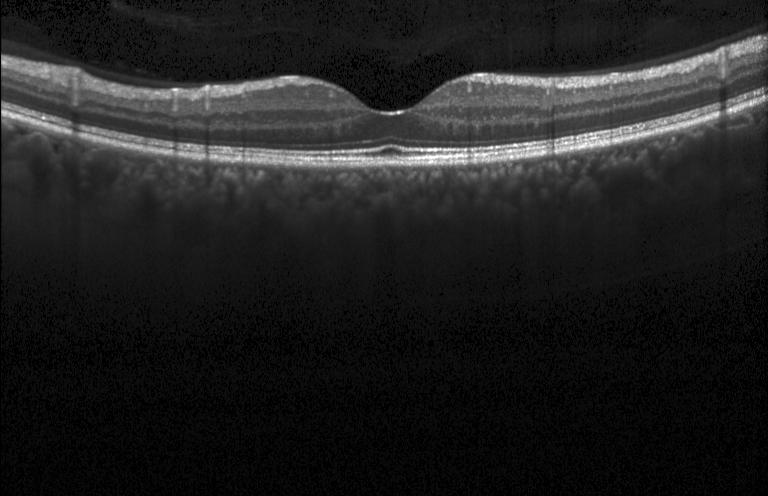 Macular scan; spectral-domain OCT; OCT line scan
Macular OCT: no choroidal neovascularization, diabetic macular edema, or drusen.